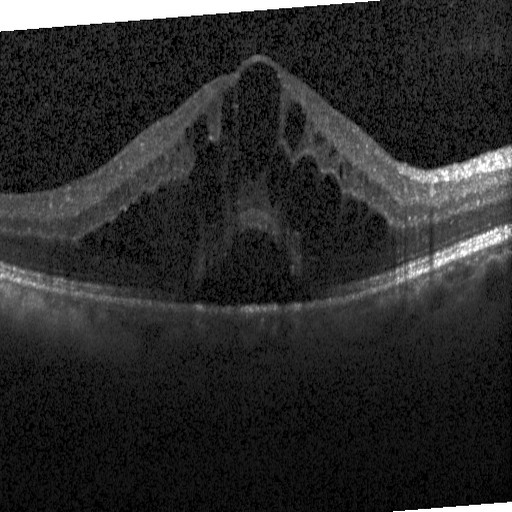

Centered on the fovea. Instrument: Heidelberg Spectralis. Retinal OCT B-scan. Spectral-domain OCT.
Diagnosis: diabetic macular edema (DME).